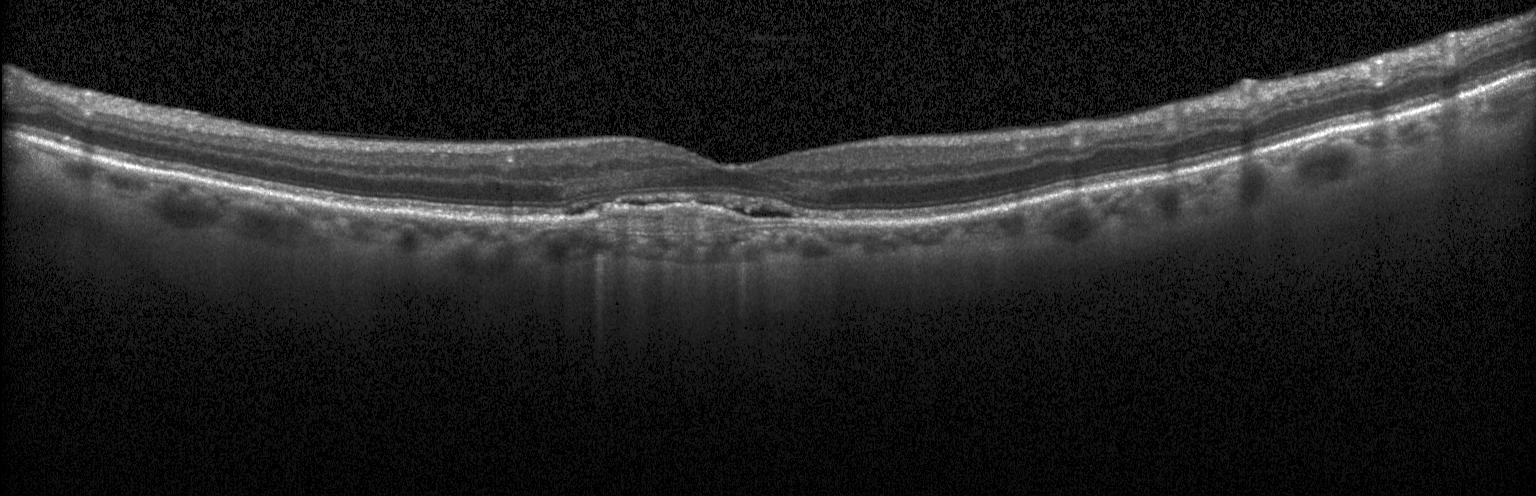 This B-scan demonstrates CNV.